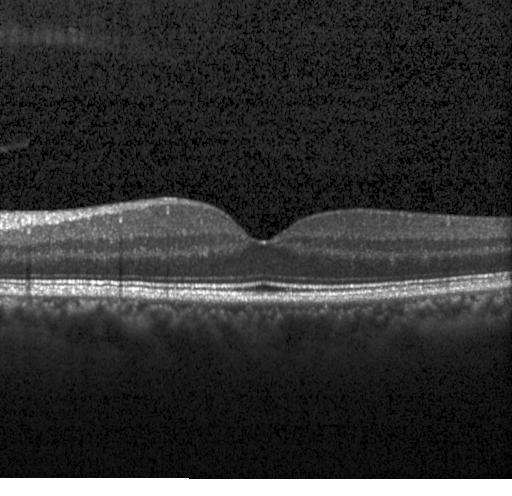
OCT line scan. Centered on the fovea. Spectral-domain OCT. The scan shows no choroidal neovascularization, no diabetic macular edema, and no drusen.